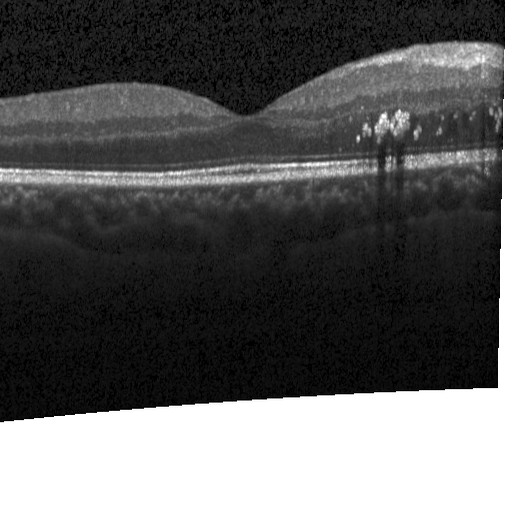
Diagnosis: diabetic macular edema.